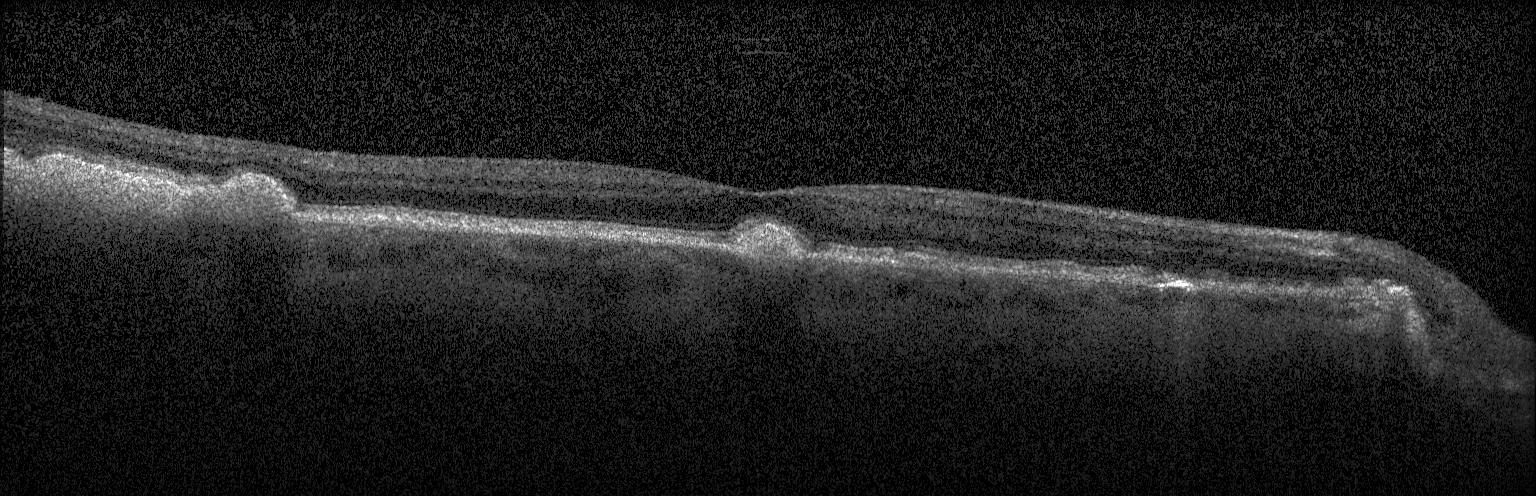 Spectral-domain OCT · fovea-centered · retinal OCT cross-section.
Diagnosis: drusen.